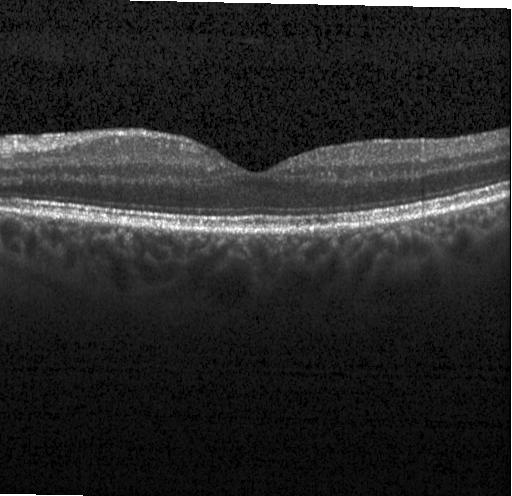
Macular OCT demonstrating no CNV, no DME, and no drusen.